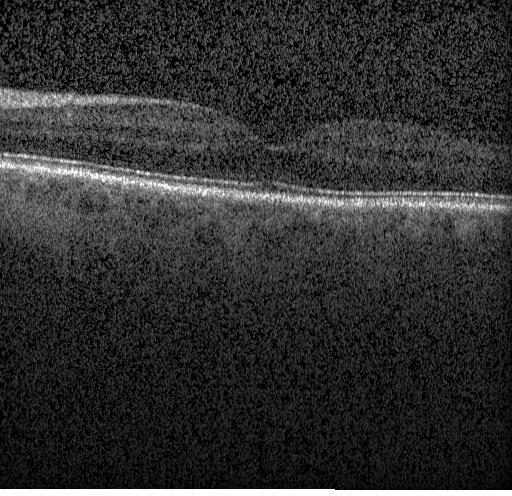

Macular OCT demonstrating no choroidal neovascularization, diabetic macular edema, or drusen.